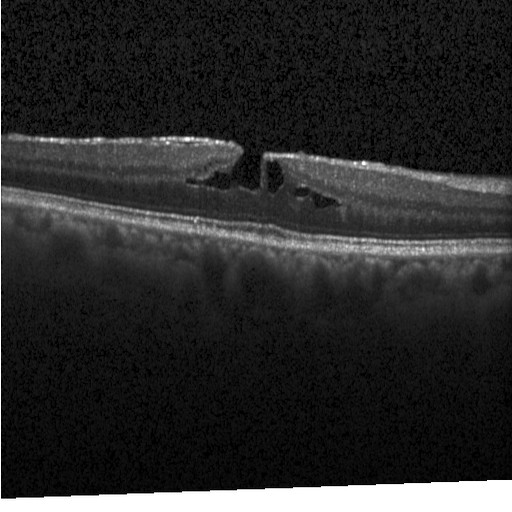
OCT line scan. Heidelberg Spectralis OCT system. Spectral-domain optical coherence tomography — The scan shows diabetic macular edema.